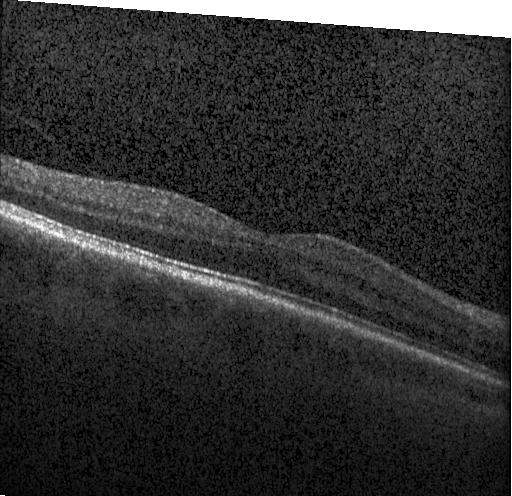

Heidelberg Spectralis; optical coherence tomography B-scan; centered on the fovea.
Diagnosis: no choroidal neovascularization, diabetic macular edema, or drusen.